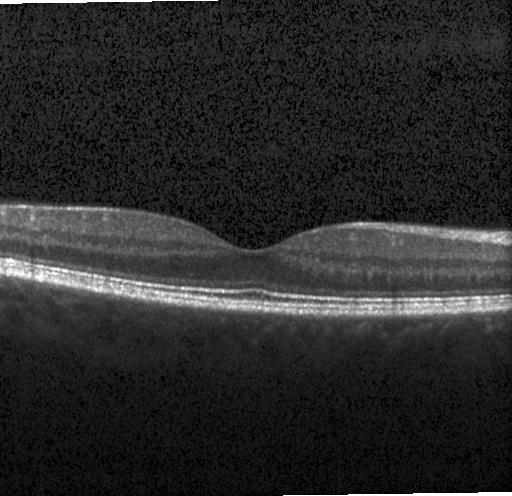 No evidence of choroidal neovascularization, diabetic macular edema, or drusen.